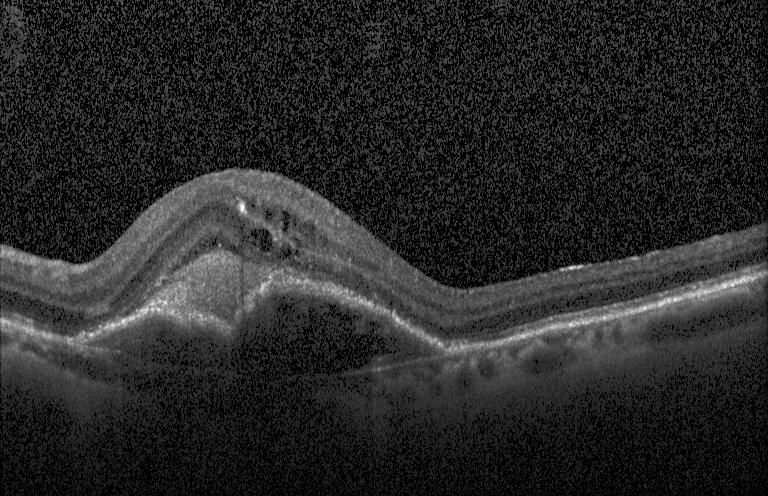

Macular scan; OCT line scan; Heidelberg Spectralis — Diagnosis: CNV.